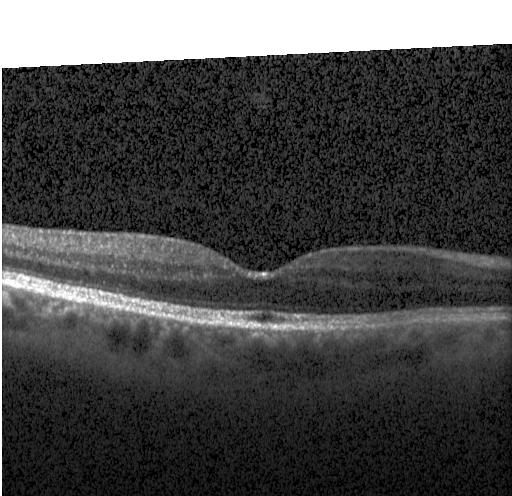

OCT finding: no evidence of choroidal neovascularization, diabetic macular edema, or drusen.